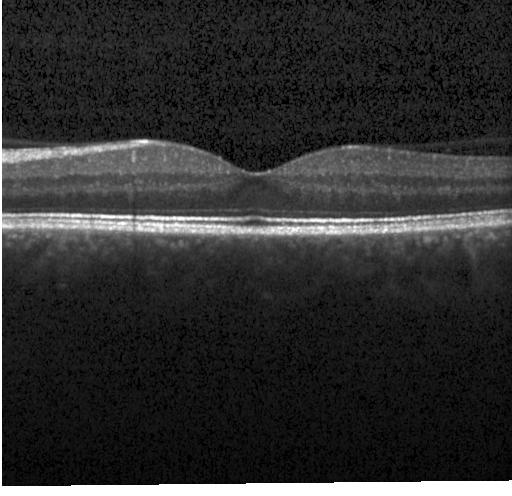 Retinal OCT B-scan; fovea-centered; Heidelberg Spectralis OCT system; spectral-domain OCT — No evidence of choroidal neovascularization, diabetic macular edema, or drusen.